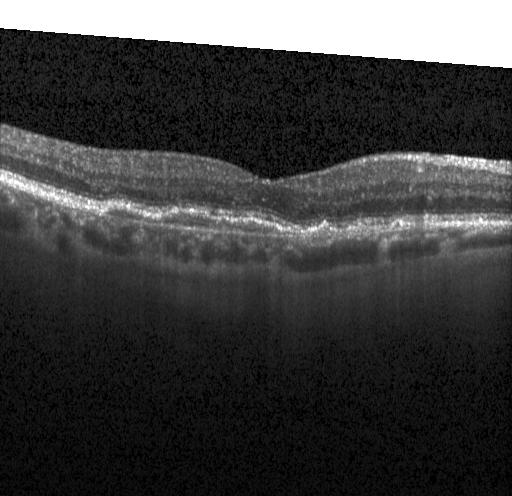
Spectral-domain optical coherence tomography, OCT B-scan. Diagnosis: CNV.